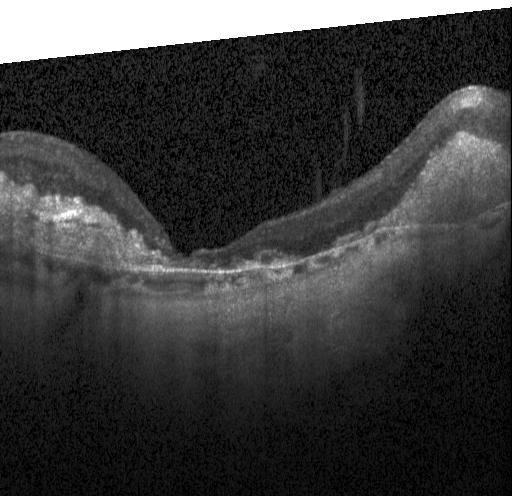

Impression: a choroidal neovascular membrane.